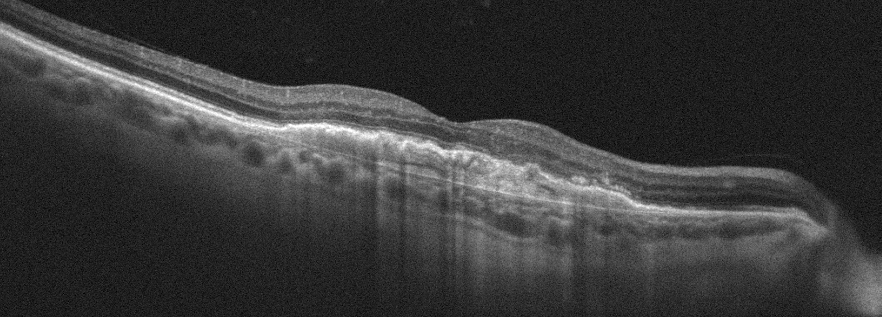 OCT B-scan; right eye
Diagnosis: age-related macular degeneration.